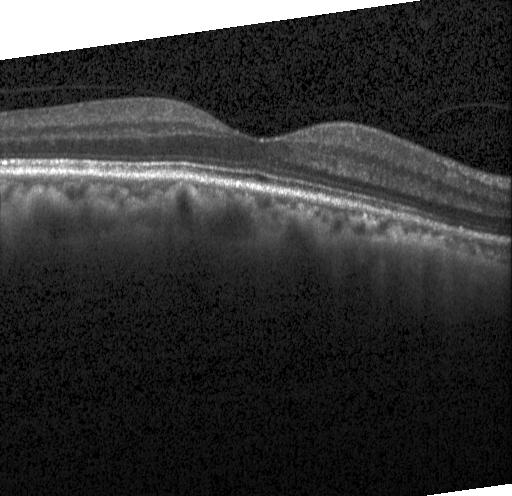

Retinal OCT B-scan, acquired on a Heidelberg Spectralis, SD-OCT — Diagnosis: no choroidal neovascularization, diabetic macular edema, or drusen.